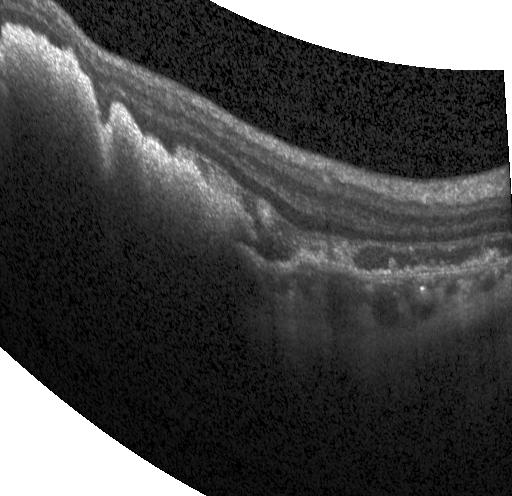

Finding: choroidal neovascularization (CNV).